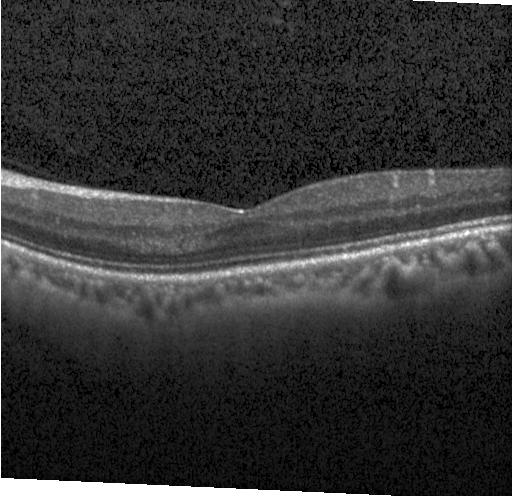
Finding: no choroidal neovascularization, no diabetic macular edema, and no drusen.